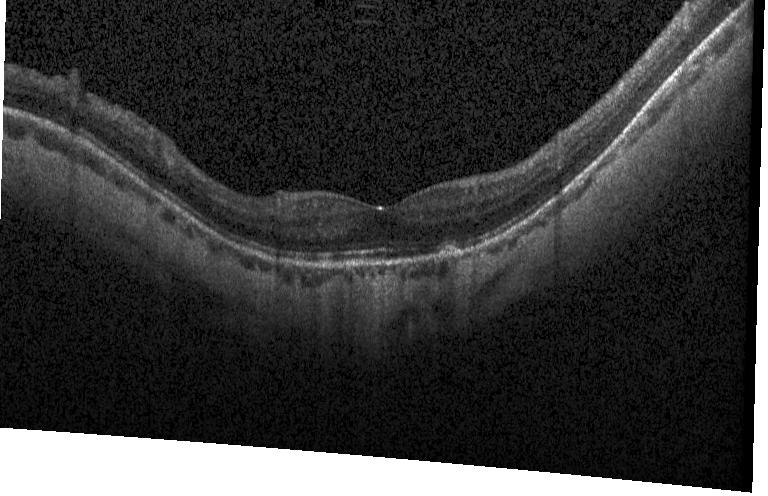
Retinal OCT B-scan, acquired on a Heidelberg Spectralis — Dx: drusen.